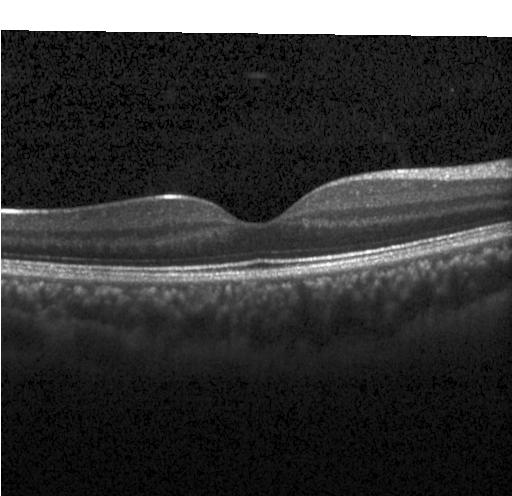 Retinal OCT B-scan — OCT finding: no choroidal neovascularization, no diabetic macular edema, and no drusen.